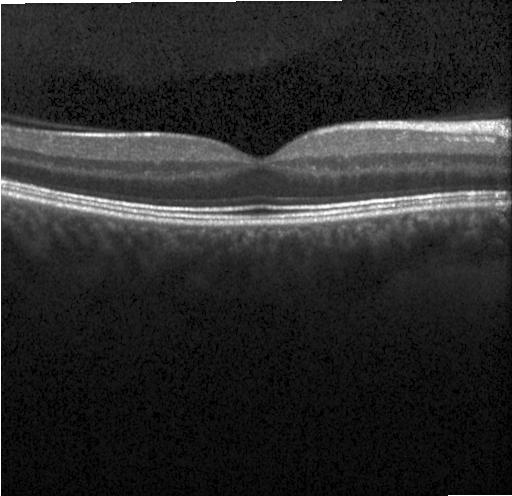 The scan shows neither choroidal neovascularization, diabetic macular edema, nor drusen.